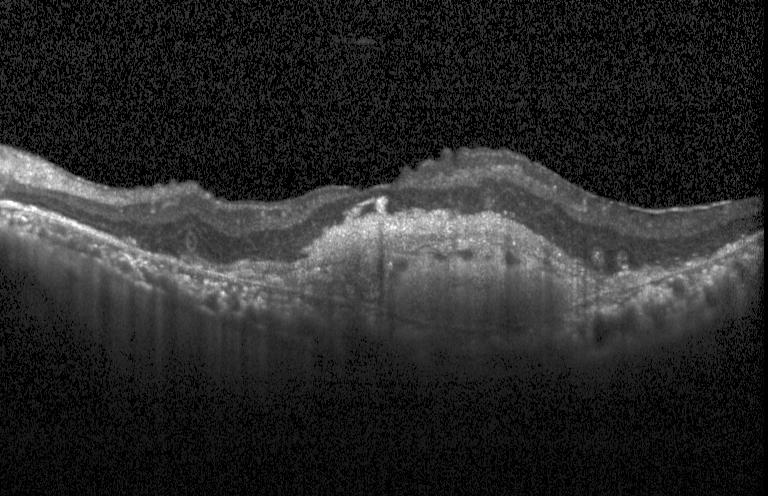
Retinal OCT cross-section — Impression: CNV.